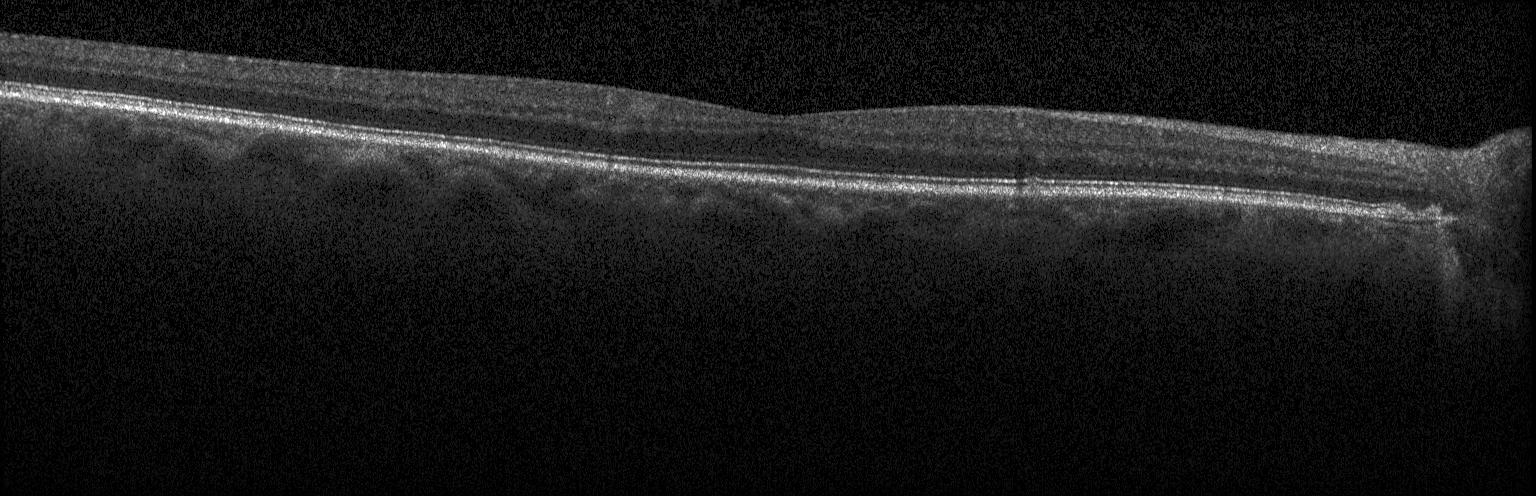 Optical coherence tomography scan — Diagnosis: no evidence of choroidal neovascularization, diabetic macular edema, or drusen.